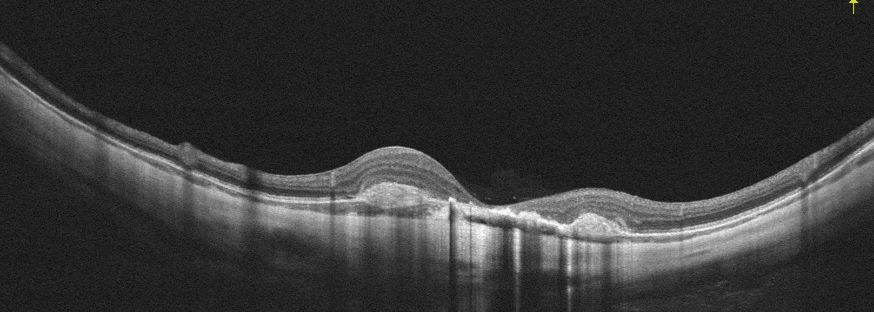

Retinal OCT B-scan
This B-scan demonstrates age-related macular degeneration.